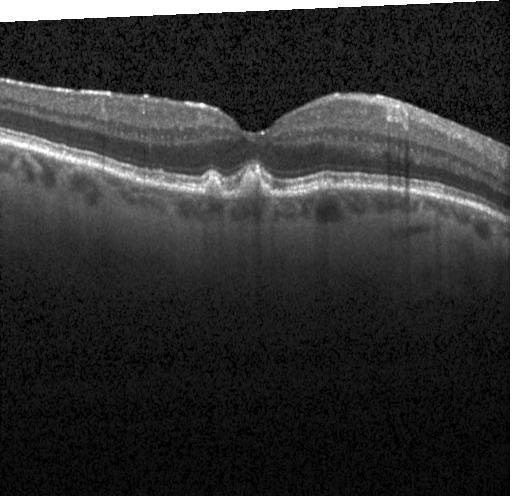
Retinal OCT B-scan, spectral-domain OCT, through the macula.
Finding: sub-RPE drusenoid deposits.